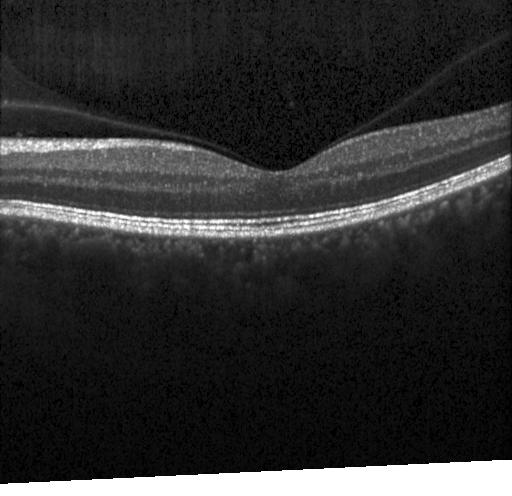 Centered on the fovea · OCT line scan · instrument: Heidelberg Spectralis.
Impression: neither choroidal neovascularization, diabetic macular edema, nor drusen.